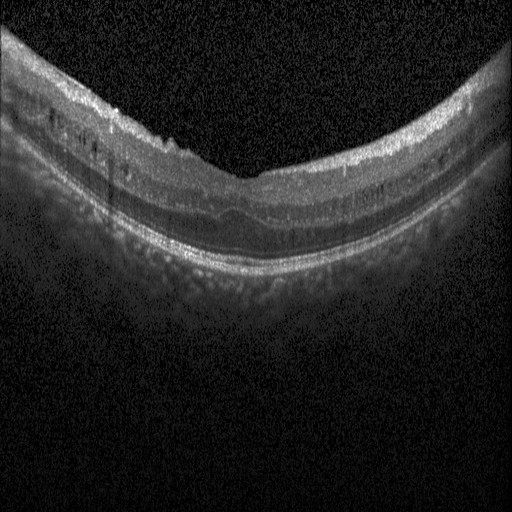 Retinal OCT B-scan — DME.